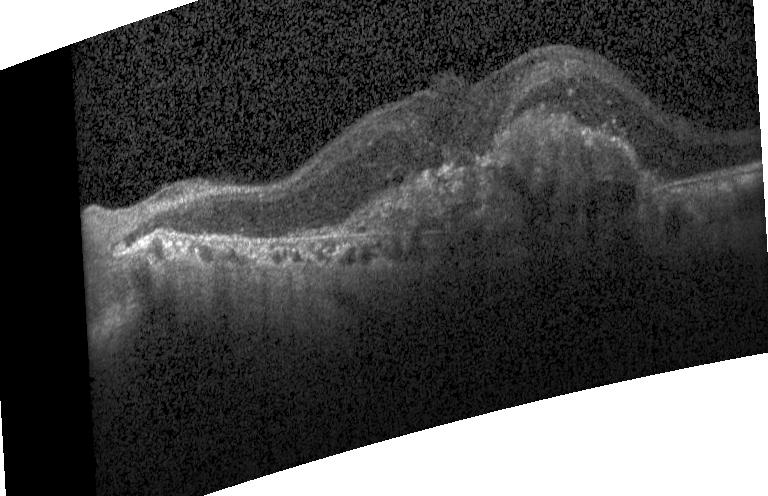

Acquired on a Heidelberg Spectralis, through the macula, spectral-domain OCT, OCT line scan — OCT finding: a choroidal neovascular membrane.